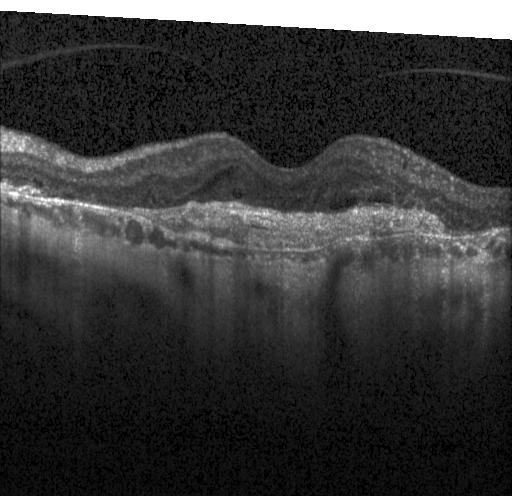

Optical coherence tomography B-scan; SD-OCT; horizontal scan through the fovea
Impression: a choroidal neovascular membrane.